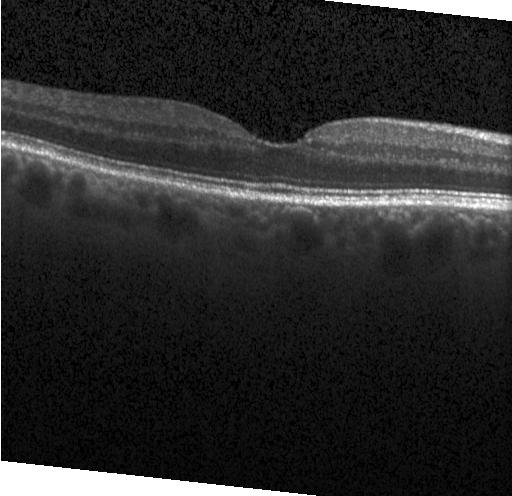 Instrument: Heidelberg Spectralis, spectral-domain OCT, OCT line scan.
Impression: no evidence of choroidal neovascularization, diabetic macular edema, or drusen.